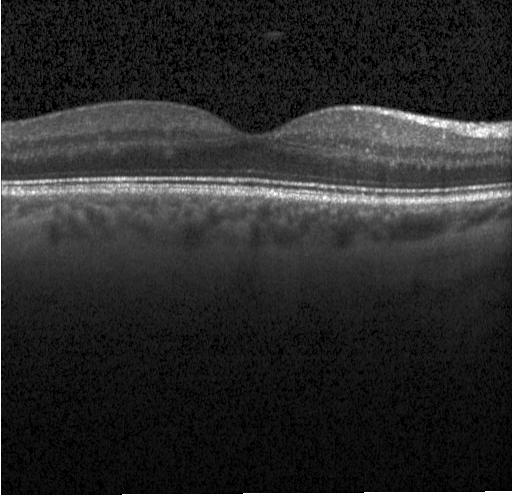 Centered on the fovea · OCT B-scan · Heidelberg Spectralis · SD-OCT.
Finding: no choroidal neovascularization, diabetic macular edema, or drusen.